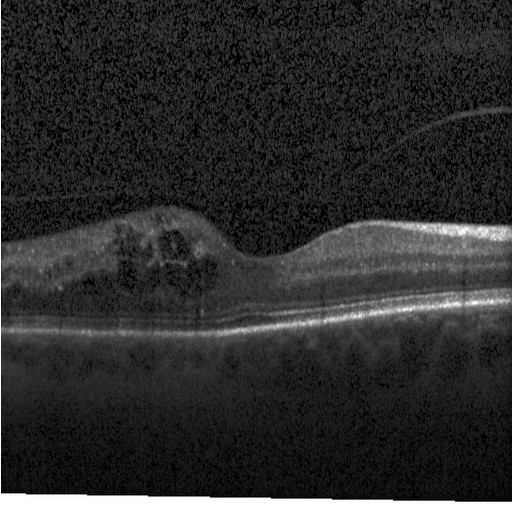
OCT B-scan showing DME.